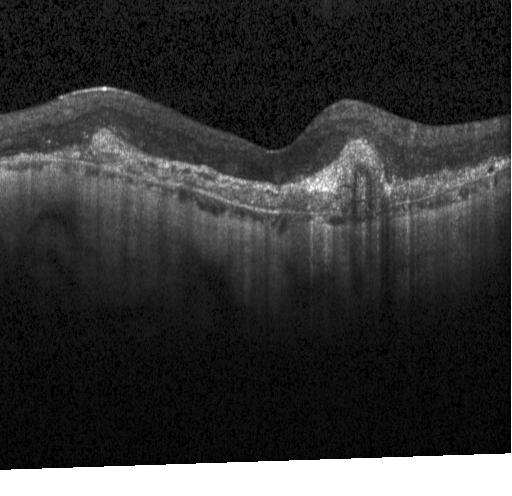 Retinal OCT cross-section showing CNV.